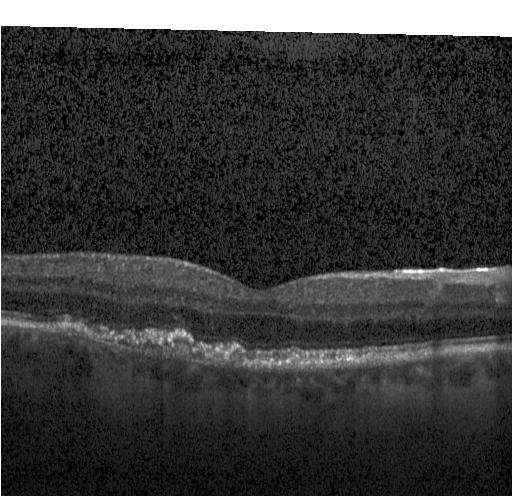 Macular scan, acquired on a Heidelberg Spectralis, OCT line scan, SD-OCT. Finding: multiple drusen.